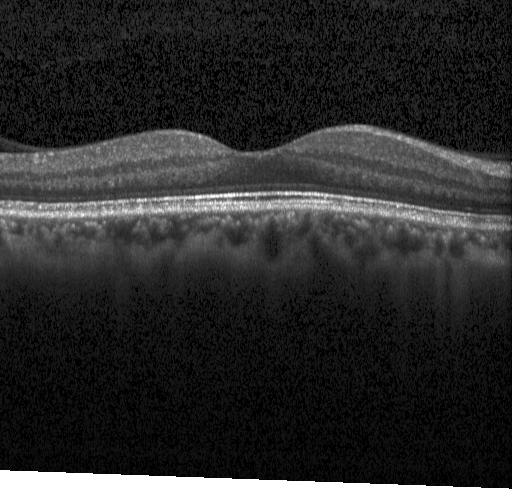

OCT line scan — Macular OCT: no choroidal neovascularization, no diabetic macular edema, and no drusen.